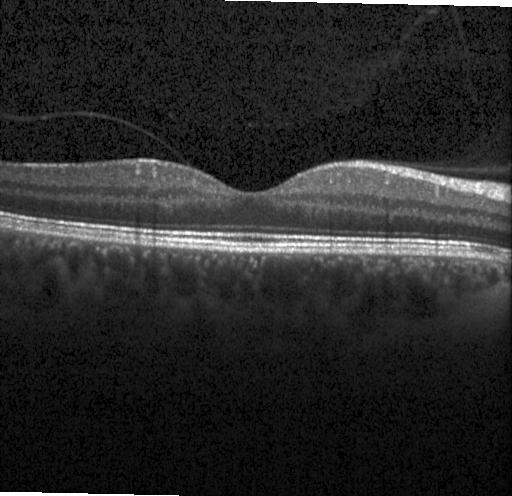 Impression: no CNV, no DME, and no drusen.